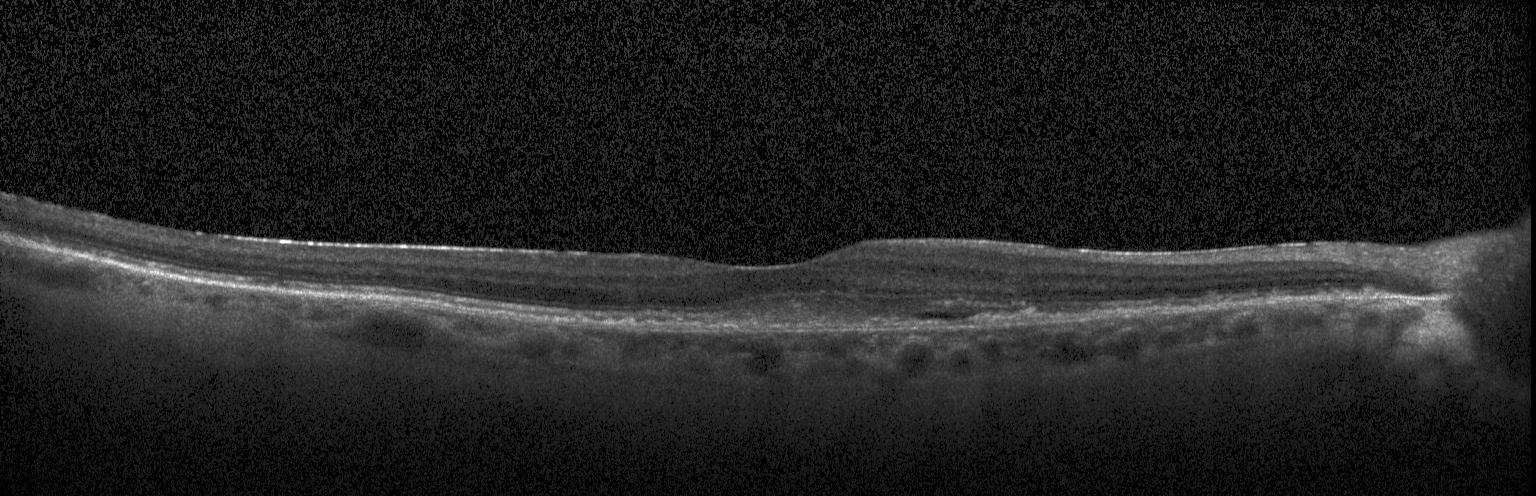
Impression: a choroidal neovascular membrane.